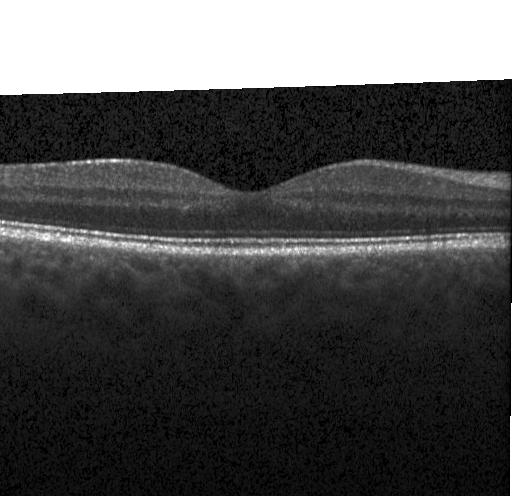 Dx: neither CNV, DME, nor drusen.